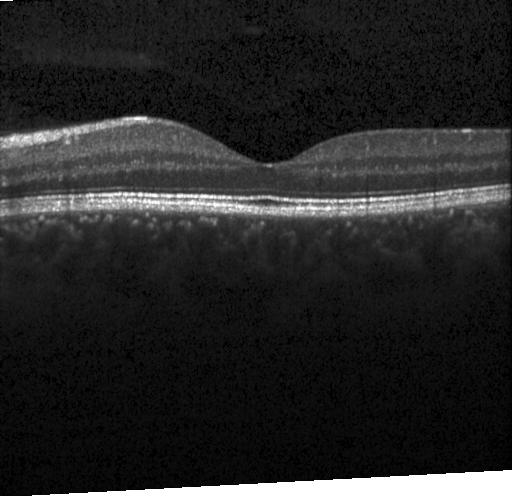
Diagnosis: no evidence of CNV, DME, or drusen.